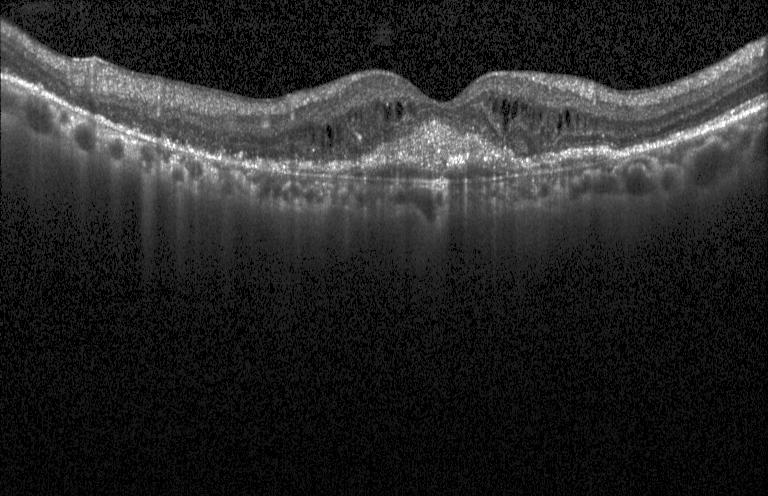

Impression: CNV.